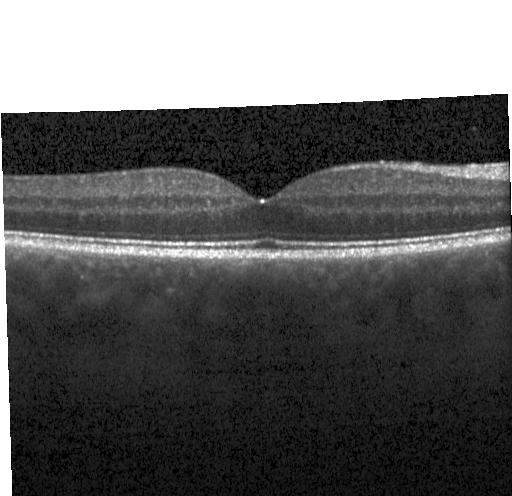
Dx: neither choroidal neovascularization, diabetic macular edema, nor drusen.